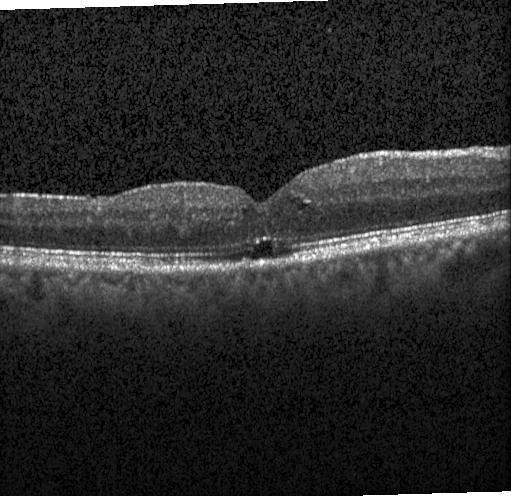

OCT B-scan showing DME.